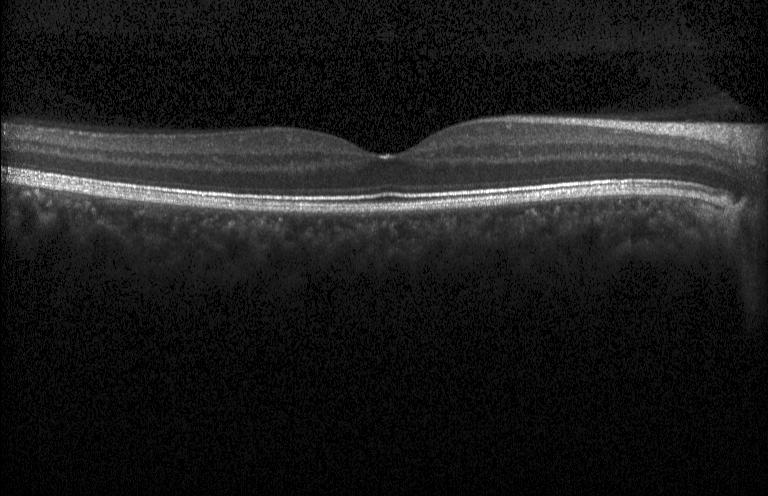 OCT B-scan, spectral-domain OCT, through the macula
The scan shows no evidence of choroidal neovascularization, diabetic macular edema, or drusen.